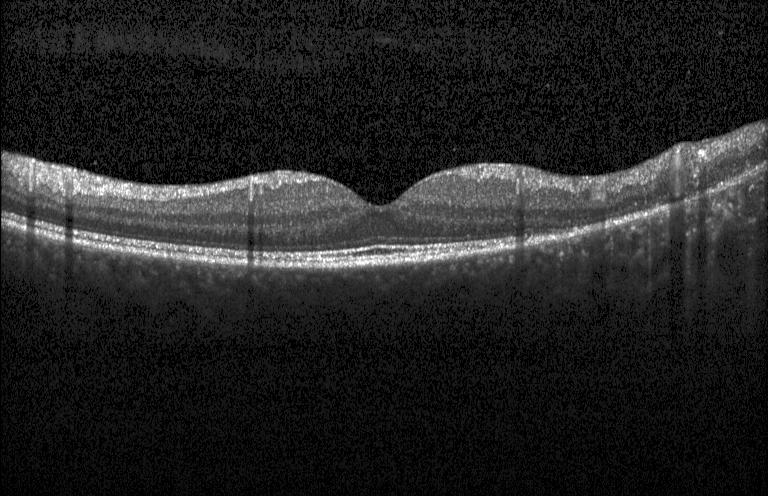 Diagnosis: neither choroidal neovascularization, diabetic macular edema, nor drusen.